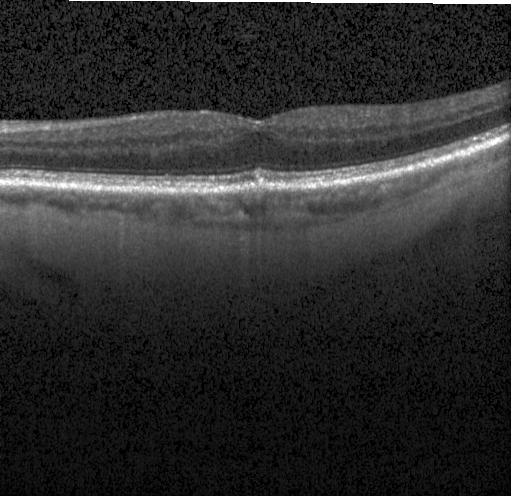

OCT B-scan showing no choroidal neovascularization, diabetic macular edema, or drusen.